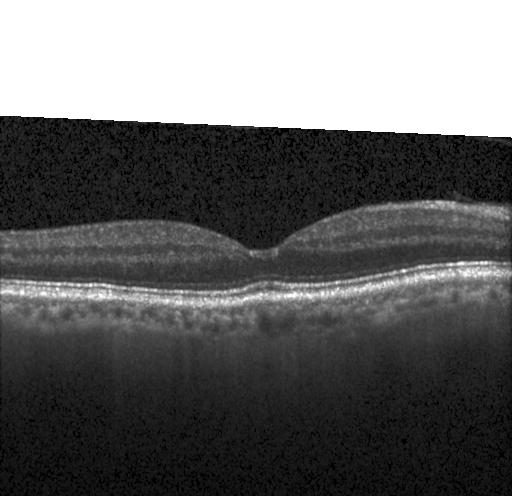

OCT B-scan showing no evidence of choroidal neovascularization, diabetic macular edema, or drusen.